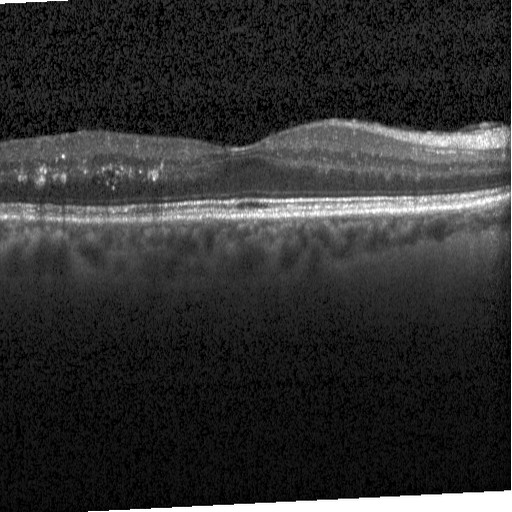
OCT B-scan; instrument: Heidelberg Spectralis.
Diabetic macular edema (DME).